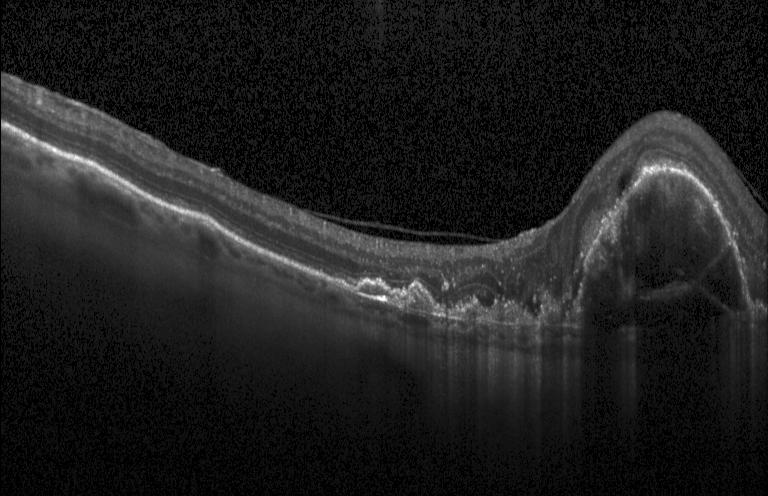 Heidelberg Spectralis. SD-OCT. OCT B-scan.
The scan shows choroidal neovascularization.